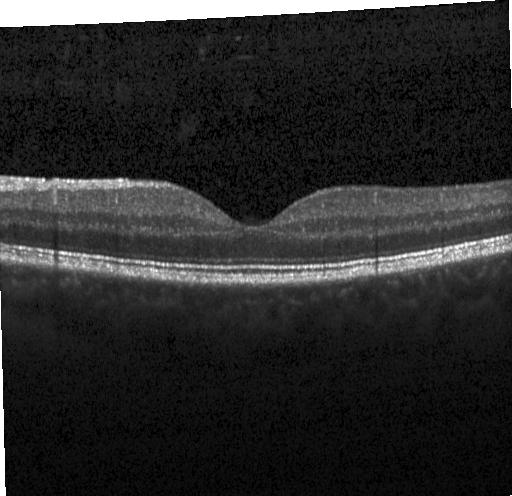
OCT B-scan. Impression: no evidence of choroidal neovascularization, diabetic macular edema, or drusen.